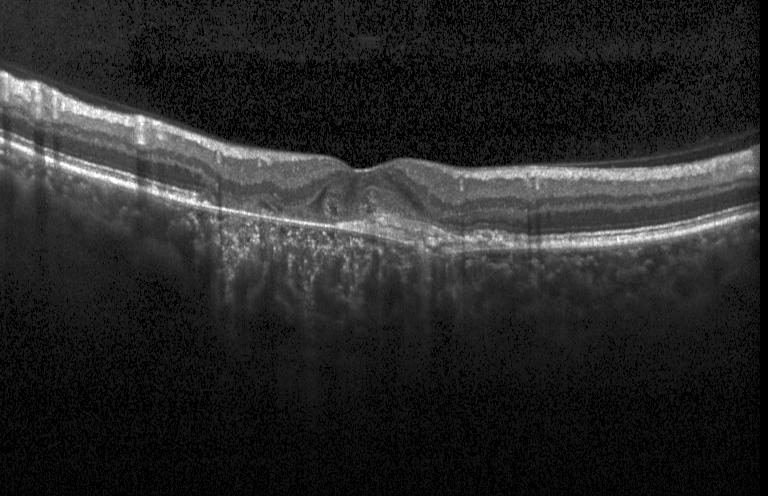
Optical coherence tomography B-scan, acquired on a Heidelberg Spectralis, through the macula, SD-OCT — Impression: choroidal neovascularization.